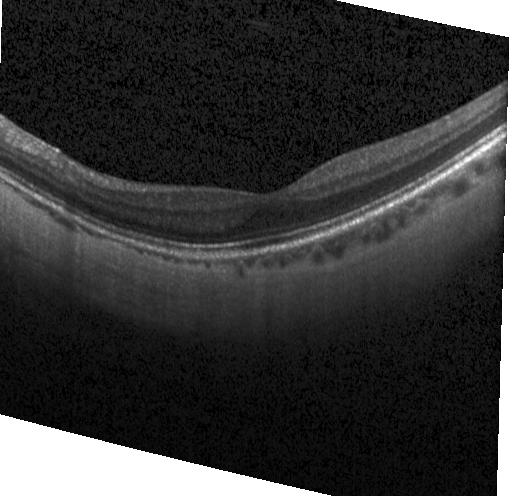
Impression: no CNV, no DME, and no drusen.